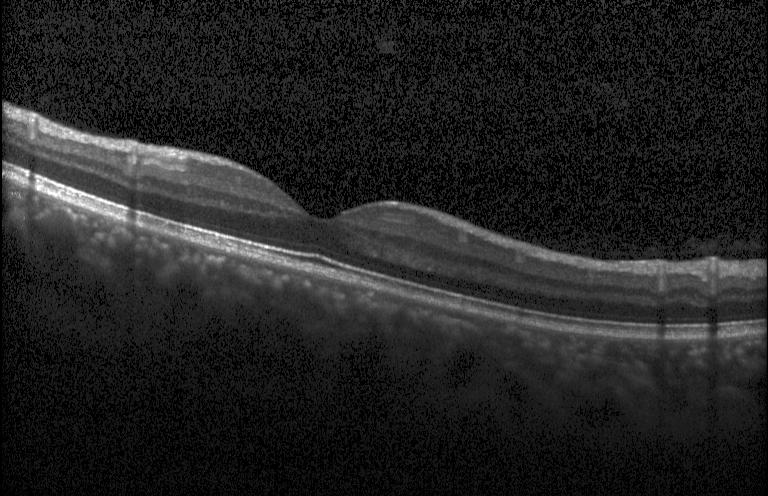

OCT B-scan, instrument: Heidelberg Spectralis, fovea-centered. Diagnosis: no choroidal neovascularization, diabetic macular edema, or drusen.